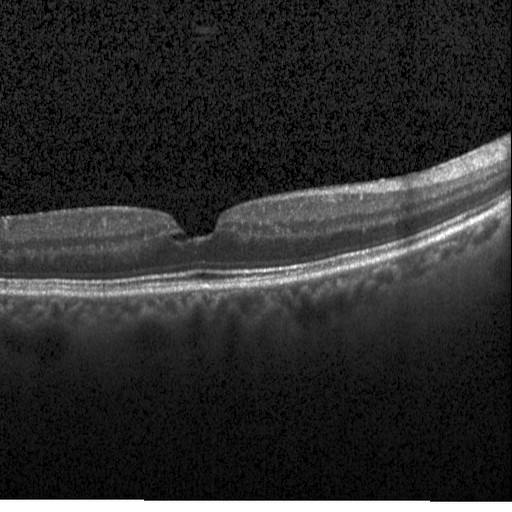
OCT B-scan showing diabetic macular edema (DME).